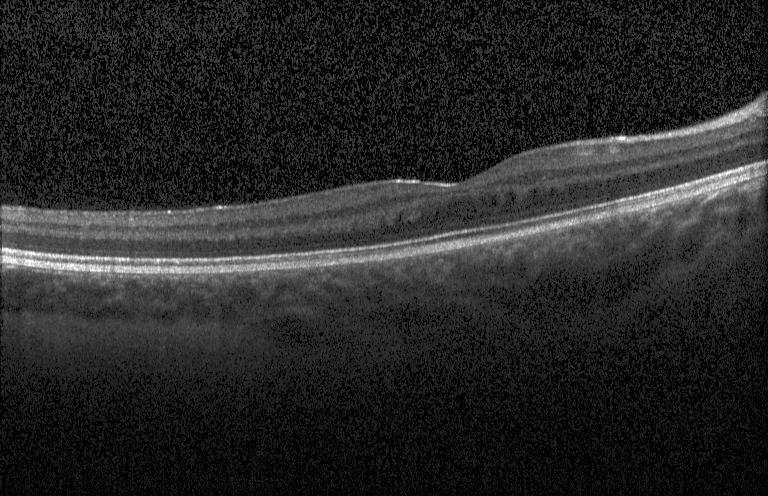
OCT line scan · Heidelberg Spectralis OCT system · centered on the fovea — Diagnosis: neither choroidal neovascularization, diabetic macular edema, nor drusen.